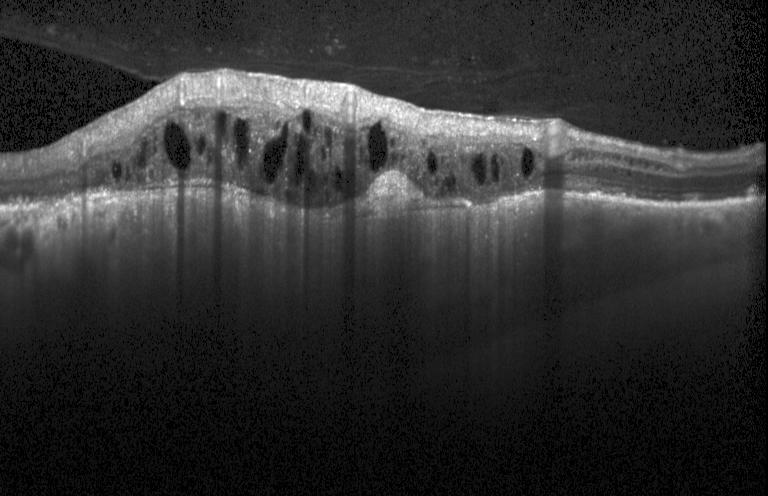
Spectral-domain OCT B-scan: a choroidal neovascular membrane.